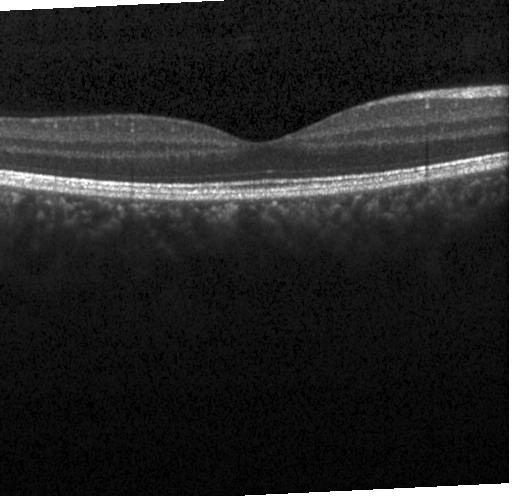
OCT line scan. Horizontal scan through the fovea. Spectral-domain OCT — This B-scan demonstrates neither CNV, DME, nor drusen.